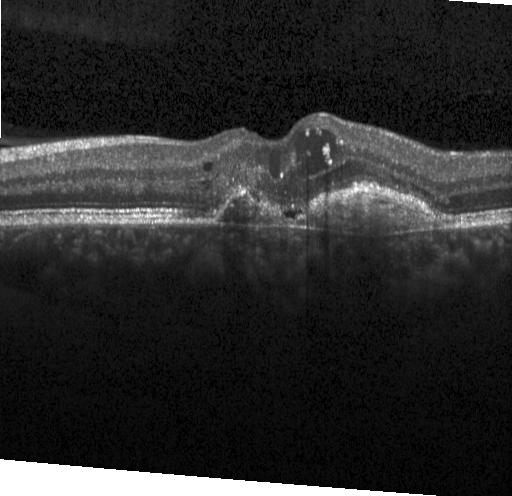 OCT B-scan showing a choroidal neovascular membrane.